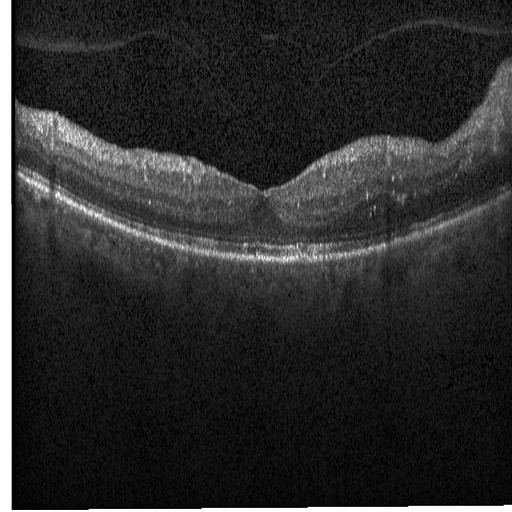 Optical coherence tomography scan
Dx: diabetic macular edema (DME).